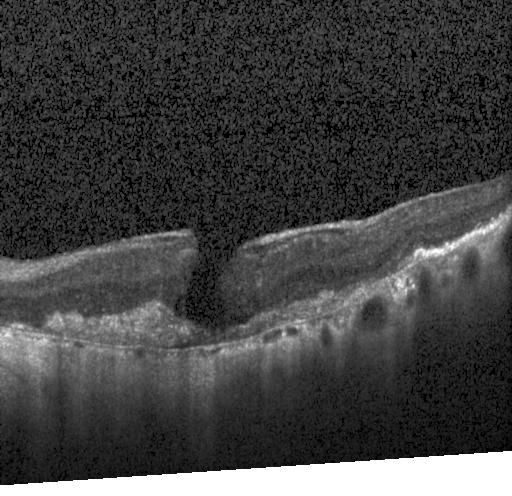

OCT B-scan showing CNV.